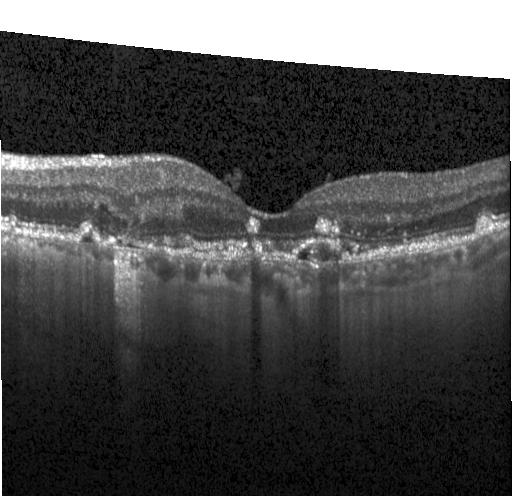 Impression: CNV.